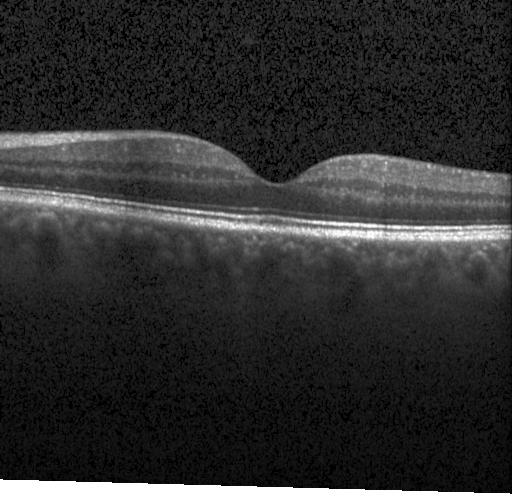
Fovea-centered · retinal OCT B-scan — Impression: no CNV, no DME, and no drusen.